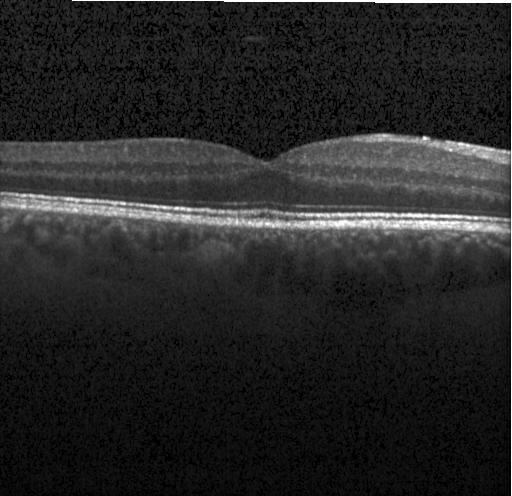 Fovea-centered · spectral-domain optical coherence tomography · optical coherence tomography B-scan. Finding: no evidence of choroidal neovascularization, diabetic macular edema, or drusen.